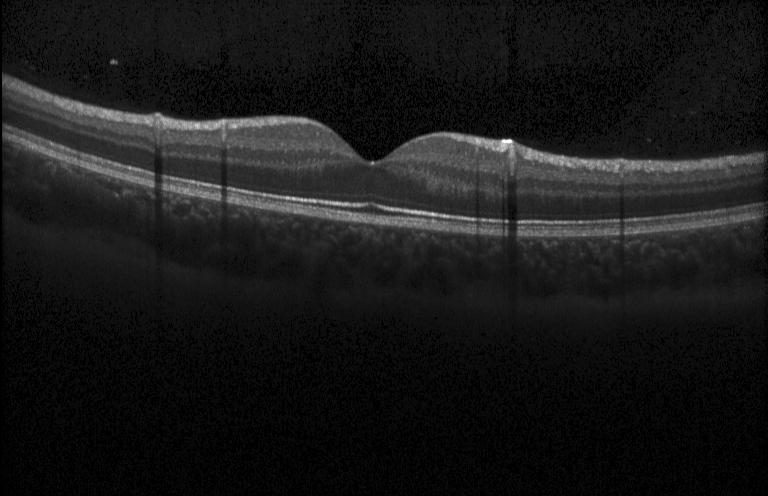

Impression: neither CNV, DME, nor drusen.